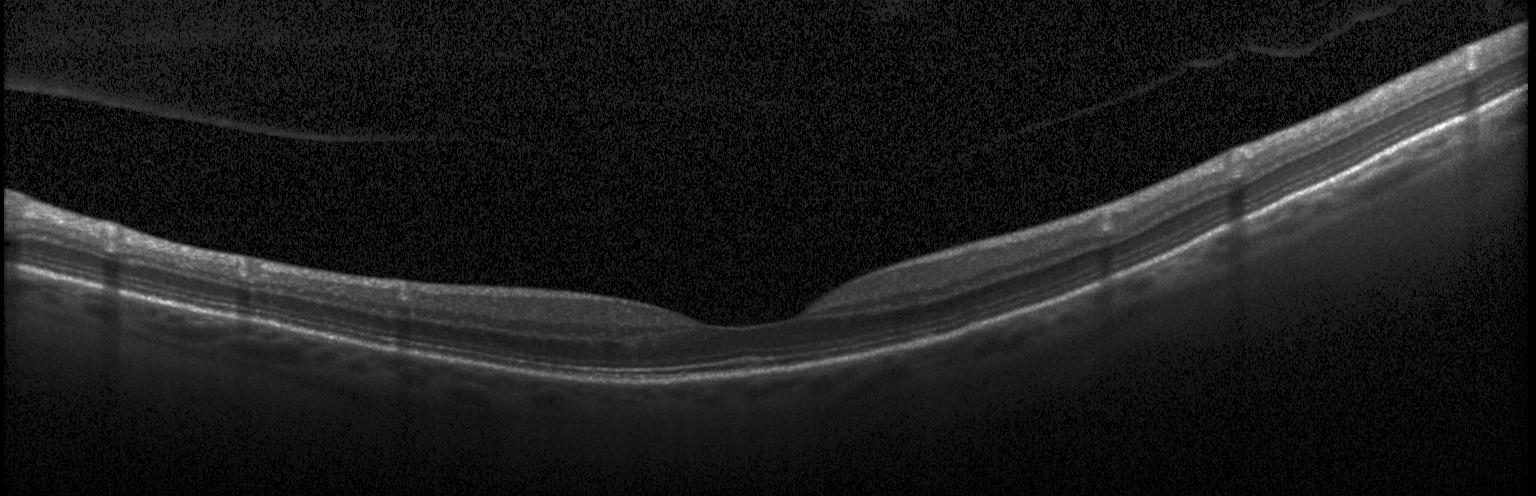 Macular scan · retinal OCT B-scan · acquired on a Heidelberg Spectralis · spectral-domain OCT
Finding: no evidence of choroidal neovascularization, diabetic macular edema, or drusen.